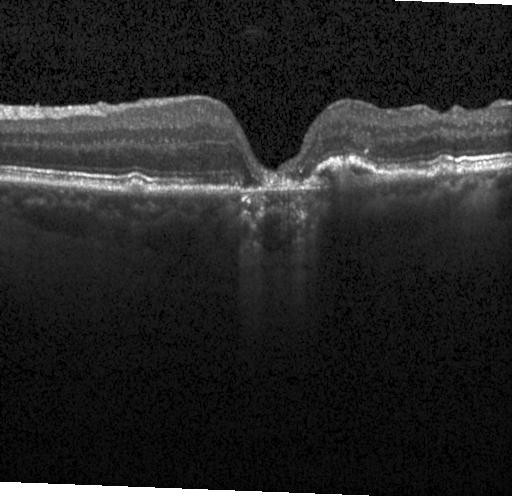 Acquired on a Heidelberg Spectralis · OCT line scan · macular scan · spectral-domain OCT.
Finding: choroidal neovascularization.